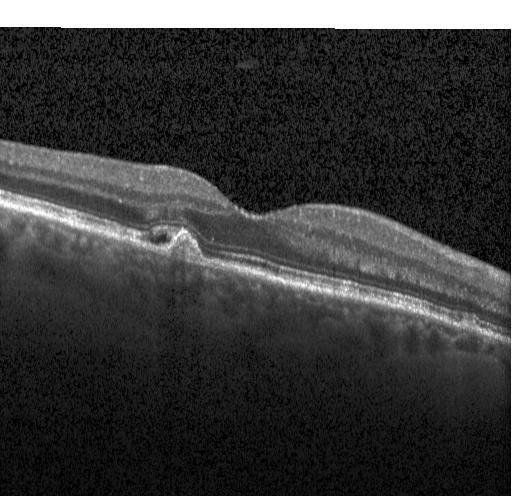
Spectral-domain OCT B-scan: choroidal neovascularization (CNV).